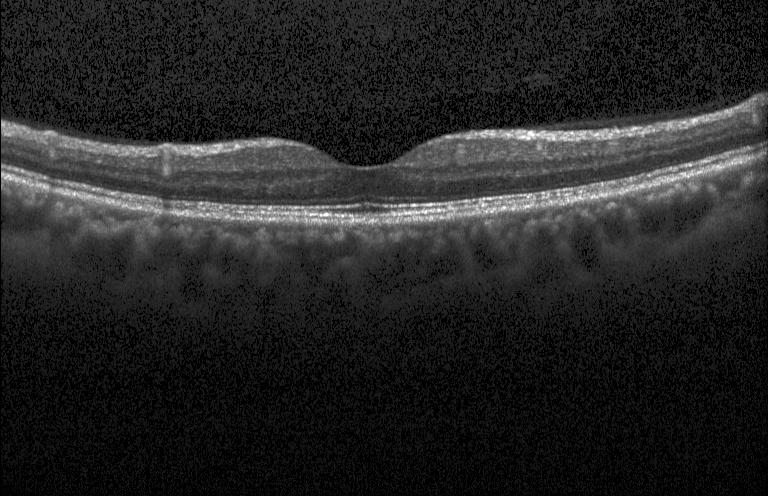
Diagnosis: no evidence of choroidal neovascularization, diabetic macular edema, or drusen.